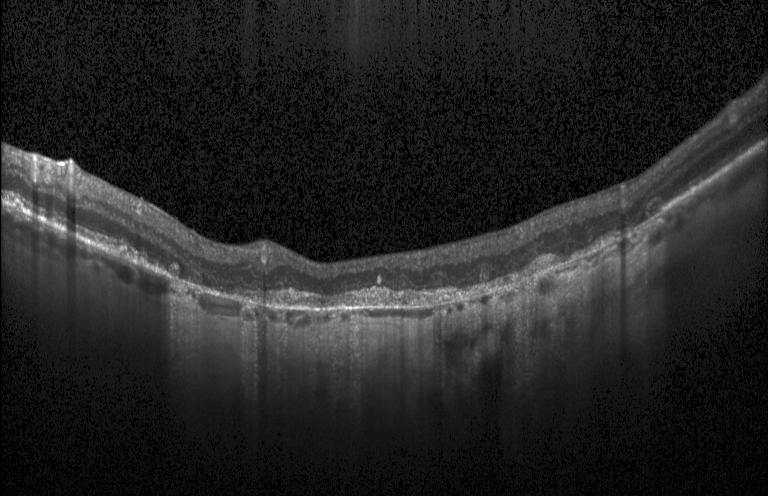 Optical coherence tomography B-scan · macular scan · SD-OCT · acquired on a Heidelberg Spectralis.
Dx: a choroidal neovascular membrane.